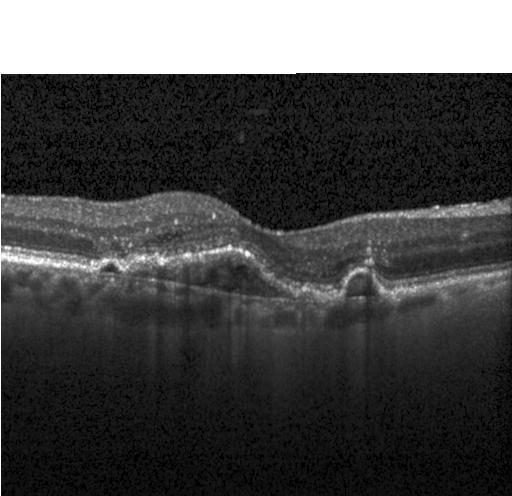
Spectral-domain OCT B-scan: a choroidal neovascular membrane.